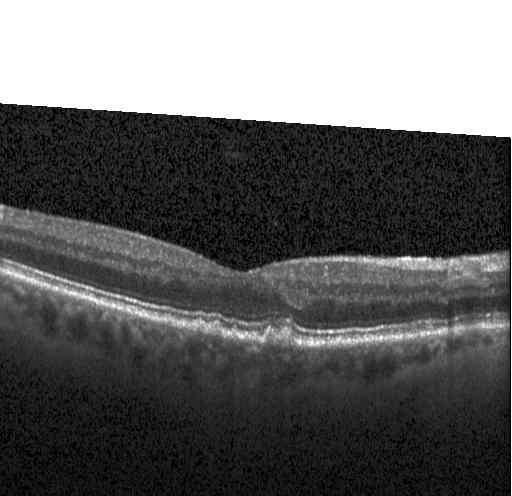

Retinal OCT cross-section showing multiple drusen.